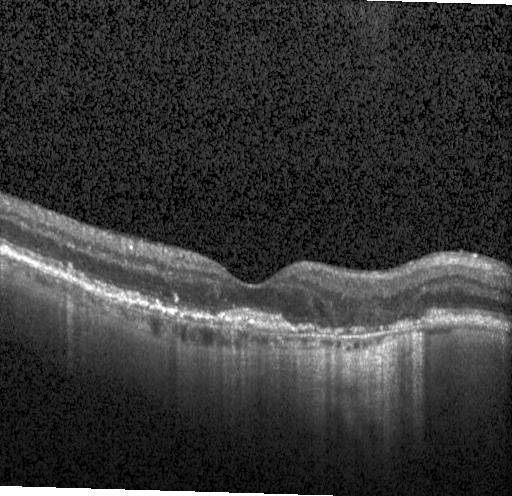
Impression: choroidal neovascularization (CNV).